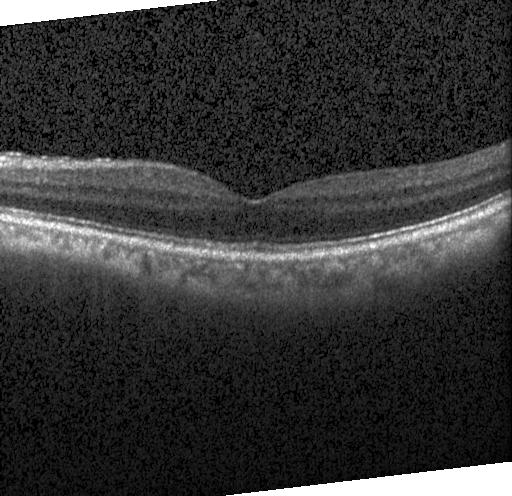
Optical coherence tomography B-scan; spectral-domain optical coherence tomography; horizontal scan through the fovea; Heidelberg Spectralis.
Diagnosis: no evidence of choroidal neovascularization, diabetic macular edema, or drusen.